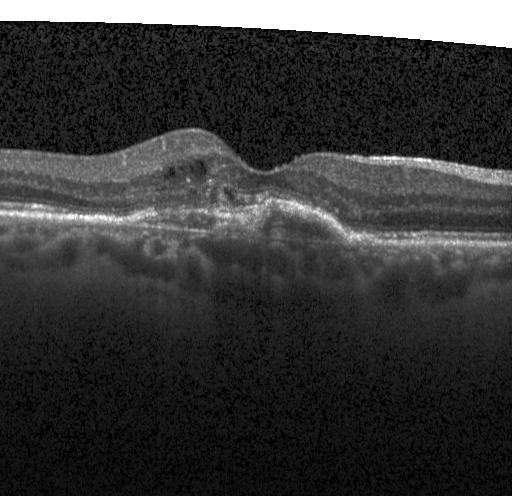 Acquired on a Heidelberg Spectralis. Optical coherence tomography scan
This B-scan demonstrates a choroidal neovascular membrane.